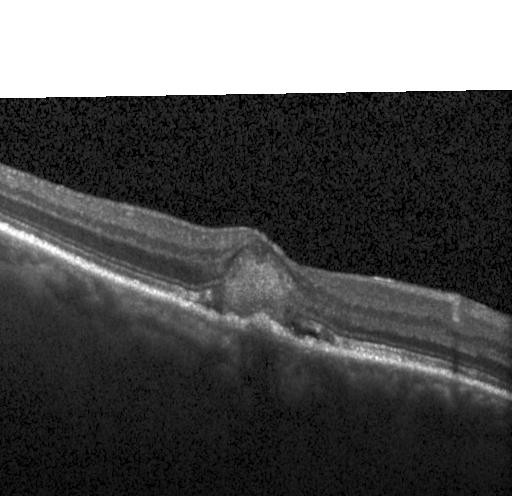

Through the macula; acquired on a Heidelberg Spectralis; spectral-domain OCT; retinal OCT cross-section.
Dx: choroidal neovascularization.